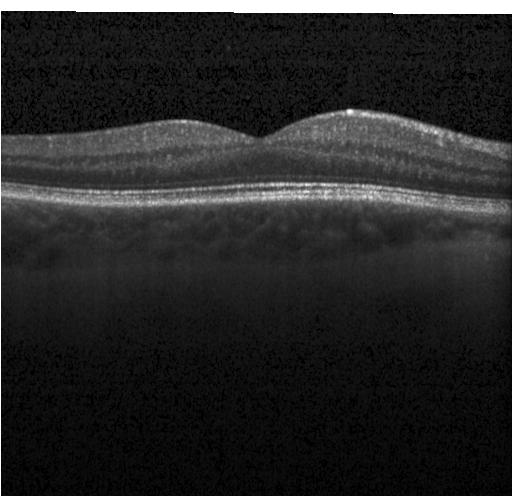
Optical coherence tomography scan · spectral-domain OCT · centered on the fovea — Diagnosis: no CNV, DME, or drusen.